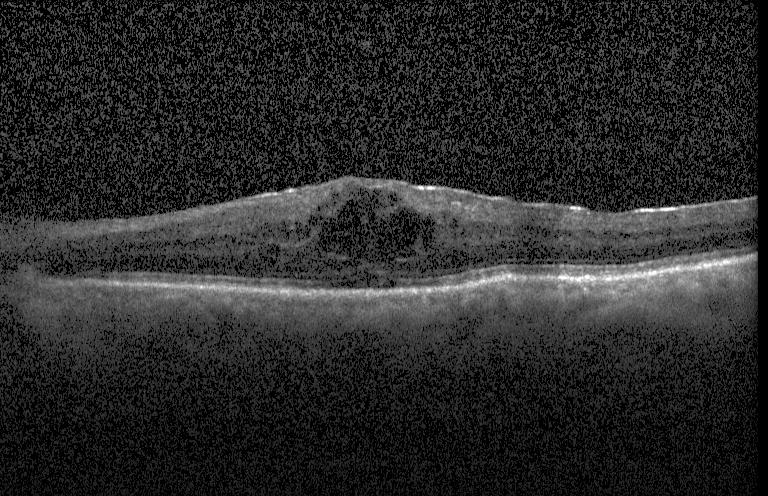 Assessment: DME.